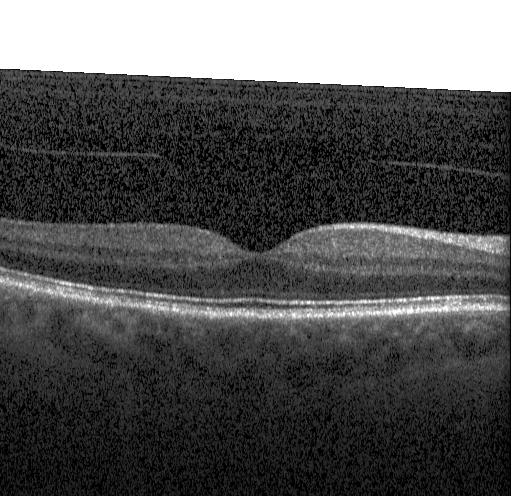

SD-OCT; instrument: Heidelberg Spectralis; OCT line scan.
Assessment: no choroidal neovascularization, no diabetic macular edema, and no drusen.